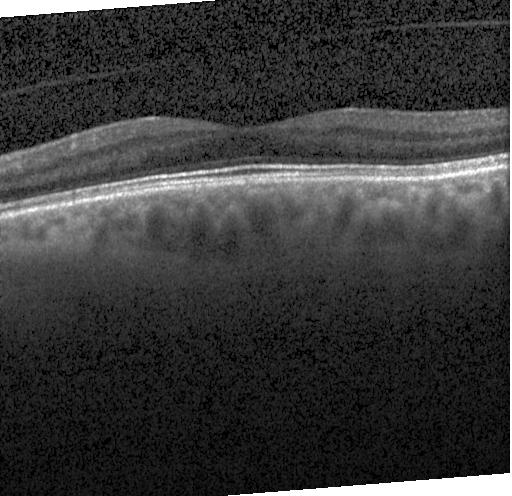 Heidelberg Spectralis, OCT B-scan, macular scan, SD-OCT — This B-scan demonstrates neither CNV, DME, nor drusen.